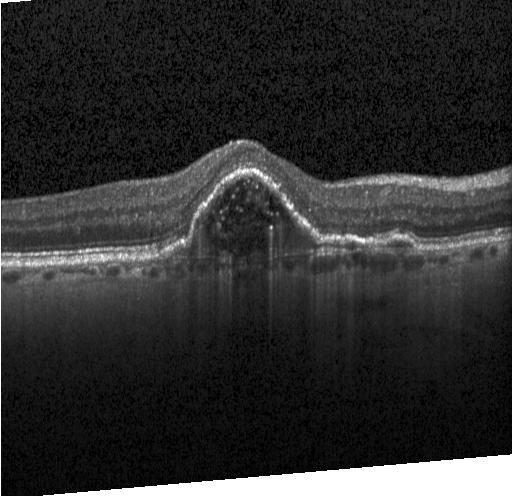

Spectral-domain optical coherence tomography; fovea-centered; optical coherence tomography scan — Diagnosis: choroidal neovascularization (CNV).